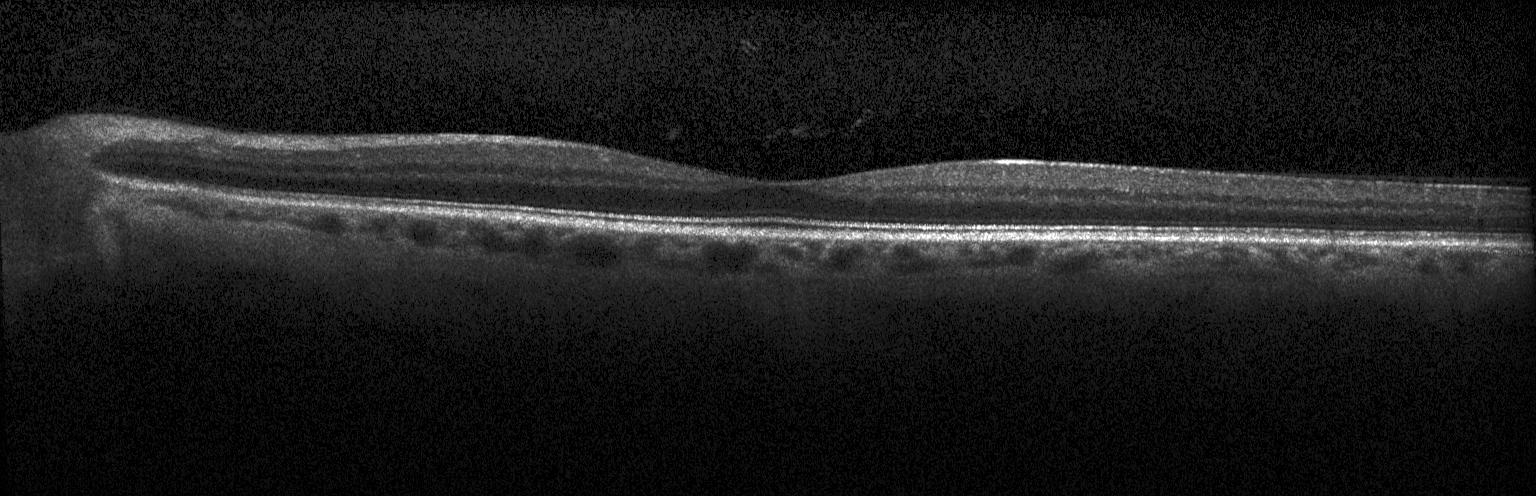 OCT finding: no choroidal neovascularization, no diabetic macular edema, and no drusen.